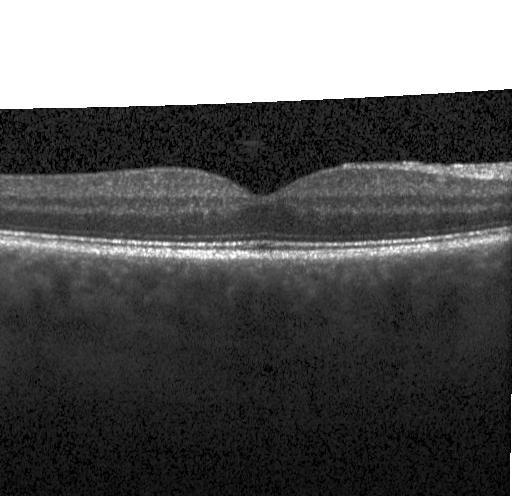
Spectral-domain OCT; optical coherence tomography B-scan; acquired on a Heidelberg Spectralis. This B-scan demonstrates no choroidal neovascularization, diabetic macular edema, or drusen.